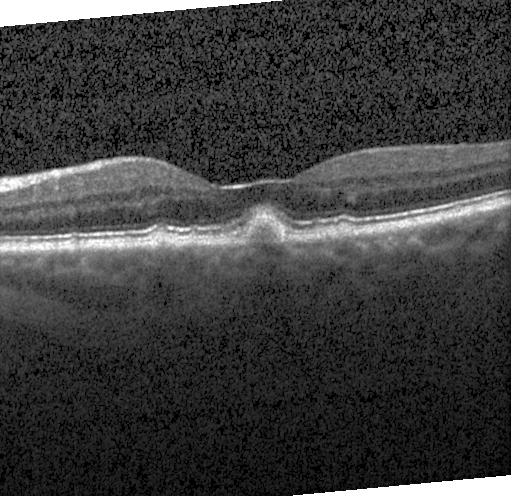
Retinal OCT cross-section showing drusen.